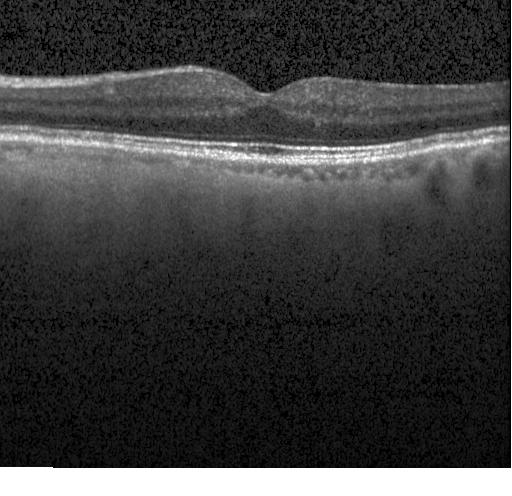 OCT finding: no evidence of choroidal neovascularization, diabetic macular edema, or drusen.